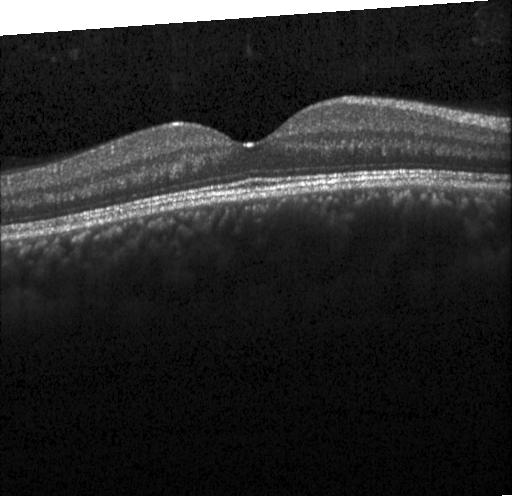
Centered on the fovea, retinal OCT cross-section, spectral-domain optical coherence tomography — OCT finding: no CNV, no DME, and no drusen.